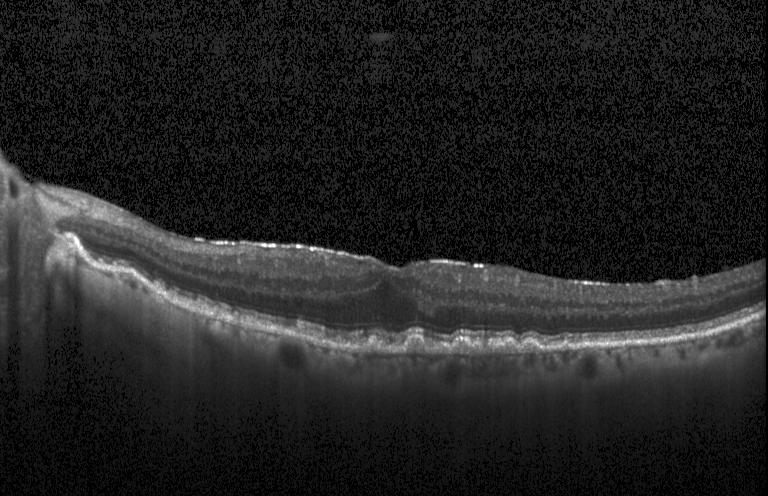

Finding: sub-RPE drusenoid deposits.